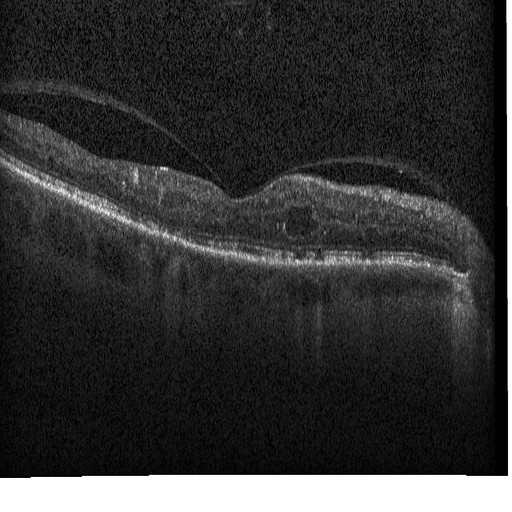

Retinal OCT cross-section showing diabetic macular edema.